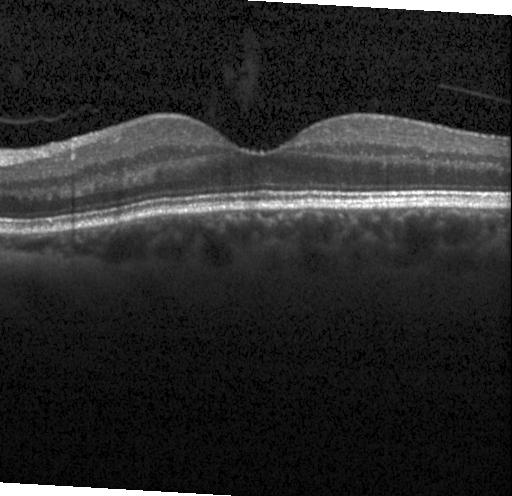

Instrument: Heidelberg Spectralis; OCT line scan — The scan shows neither CNV, DME, nor drusen.